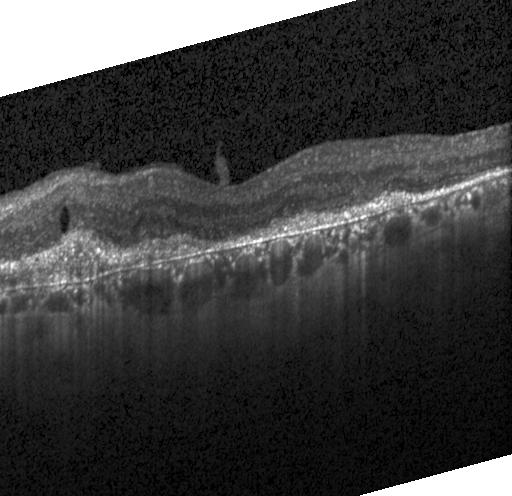
Optical coherence tomography B-scan.
Macular OCT: CNV.